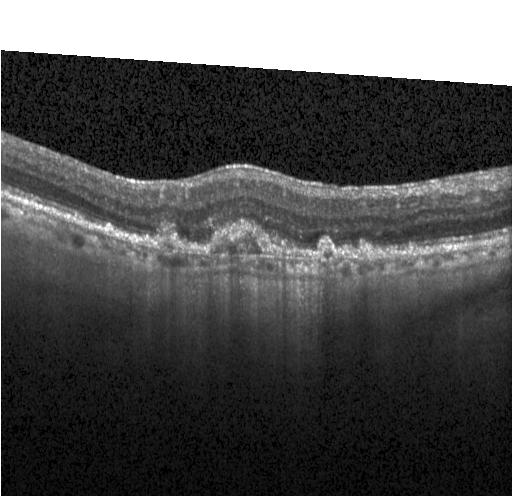 Acquired on a Heidelberg Spectralis, spectral-domain optical coherence tomography, fovea-centered, retinal OCT cross-section
Dx: choroidal neovascularization.